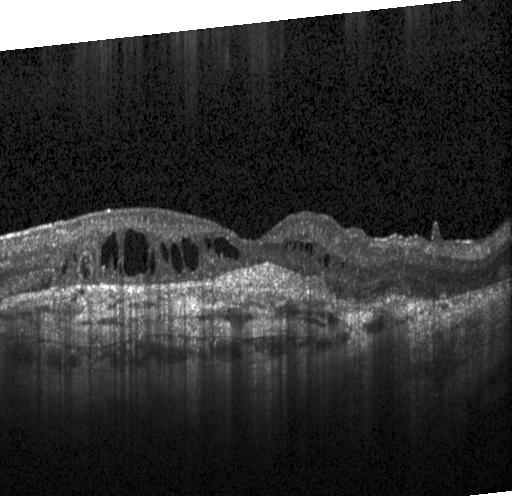 Assessment: a choroidal neovascular membrane.